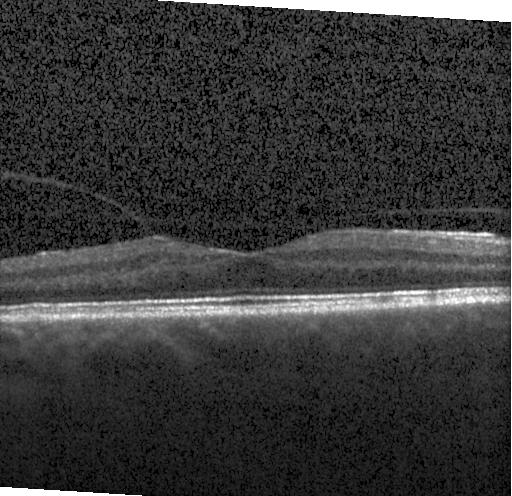 OCT line scan; spectral-domain OCT.
Assessment: no CNV, no DME, and no drusen.